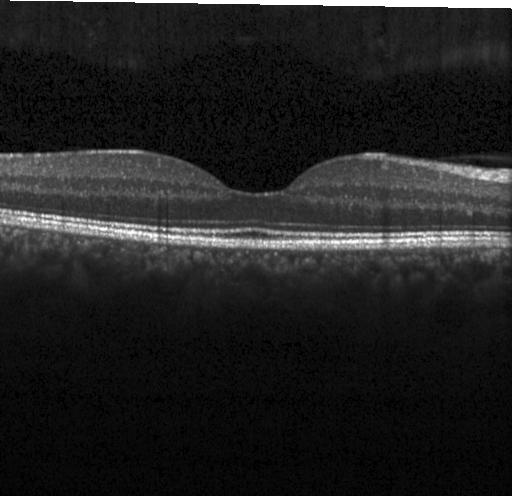

OCT line scan.
Finding: no choroidal neovascularization, diabetic macular edema, or drusen.